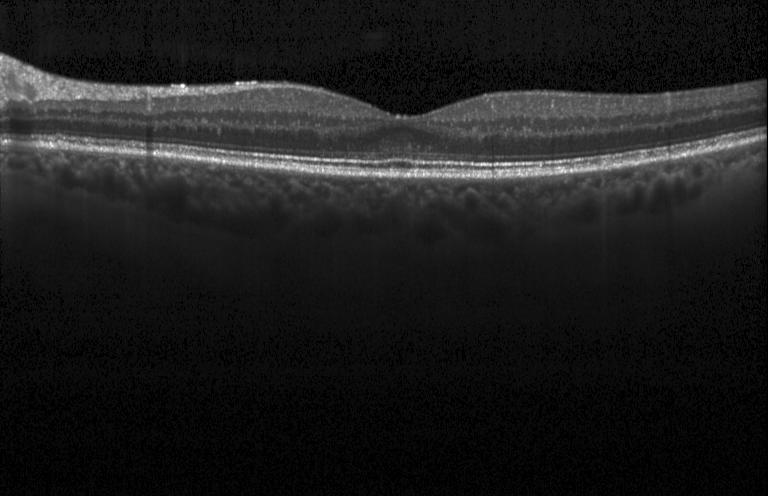
Retinal OCT B-scan — Impression: no evidence of CNV, DME, or drusen.